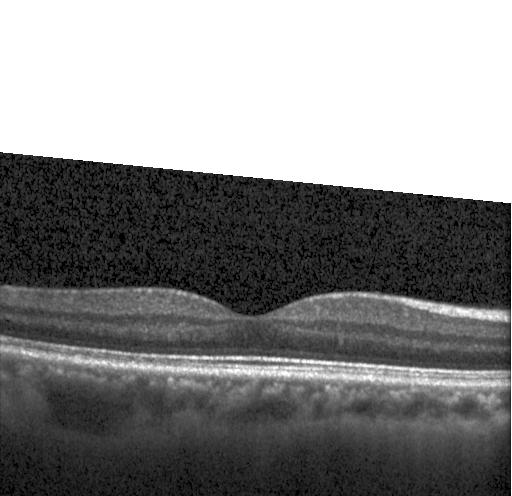
Macular OCT: no evidence of choroidal neovascularization, diabetic macular edema, or drusen.